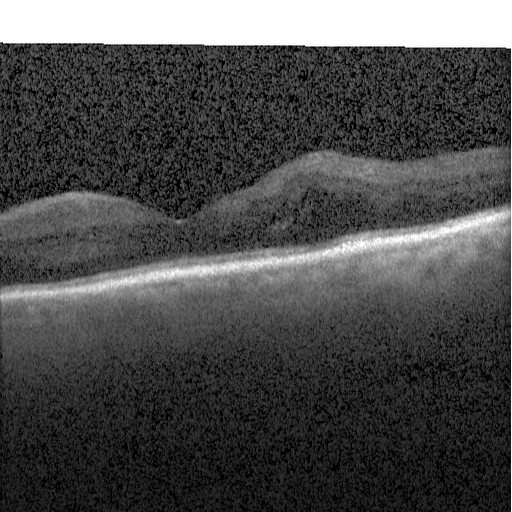

Instrument: Heidelberg Spectralis; SD-OCT; fovea-centered; optical coherence tomography B-scan. Impression: DME.